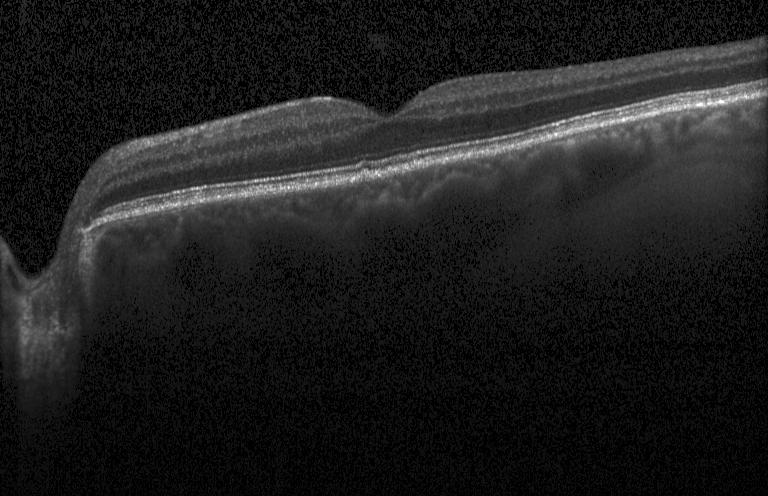

This B-scan demonstrates multiple drusen.